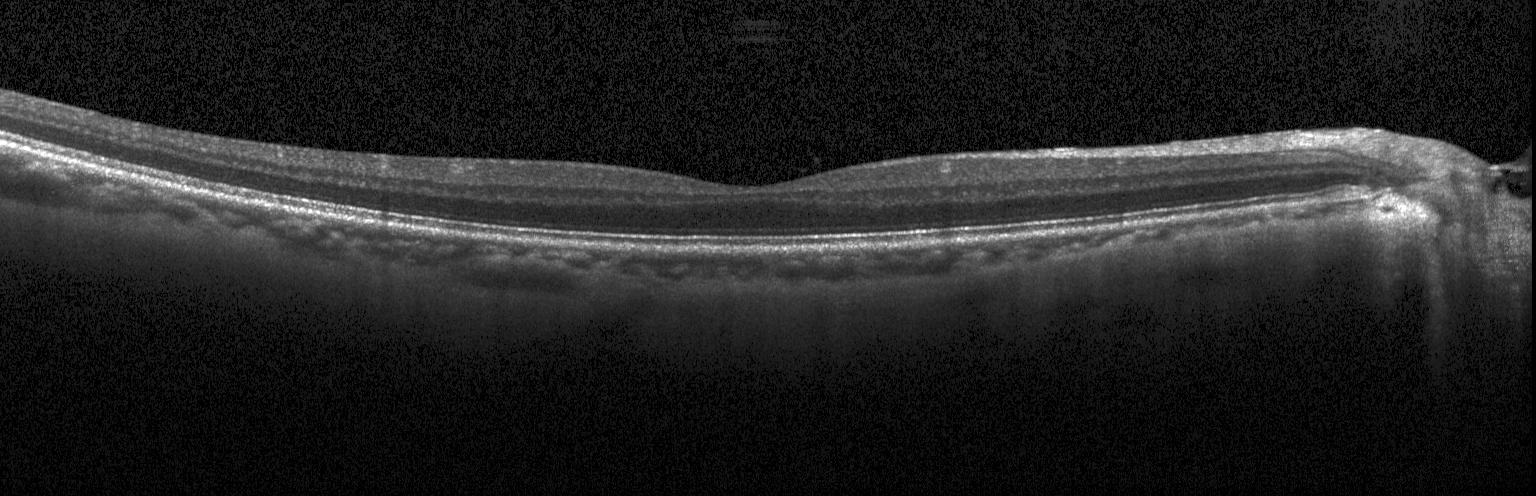 Retinal OCT B-scan — Diagnosis: no evidence of choroidal neovascularization, diabetic macular edema, or drusen.